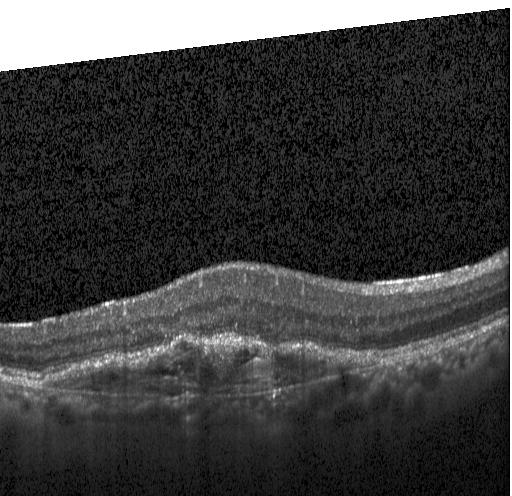 Heidelberg Spectralis OCT system · spectral-domain optical coherence tomography · centered on the fovea · retinal OCT cross-section
Diagnosis: a choroidal neovascular membrane.